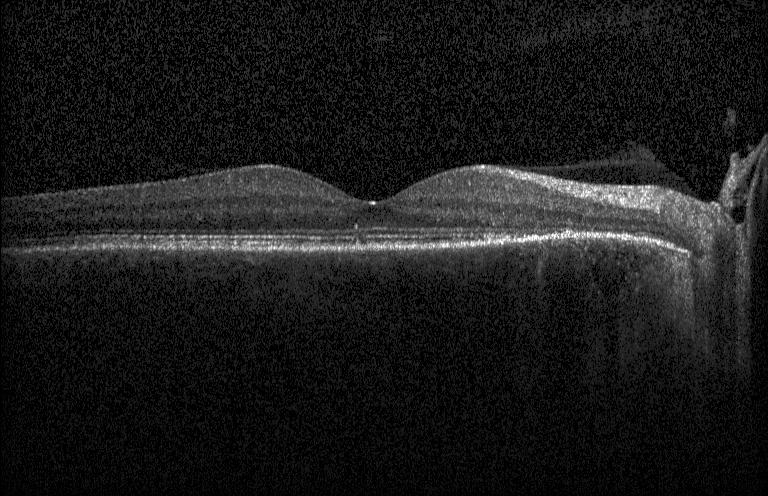

This B-scan demonstrates no choroidal neovascularization, diabetic macular edema, or drusen.